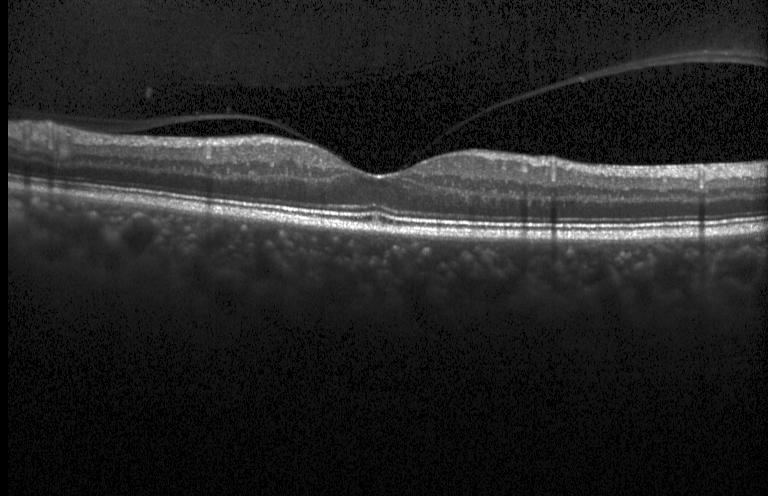
Macular OCT: no evidence of choroidal neovascularization, diabetic macular edema, or drusen.